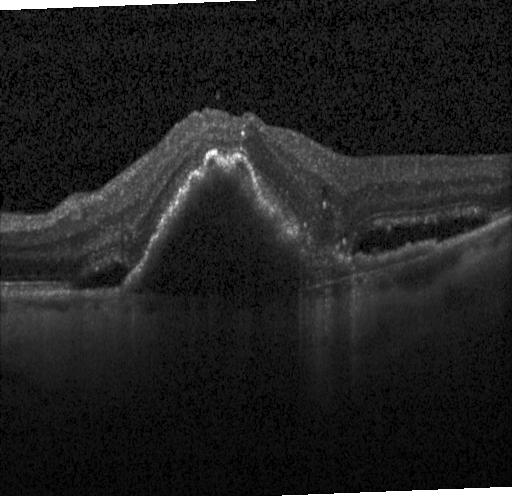 Retinal OCT B-scan; macular scan; spectral-domain optical coherence tomography; instrument: Heidelberg Spectralis — Finding: choroidal neovascularization.